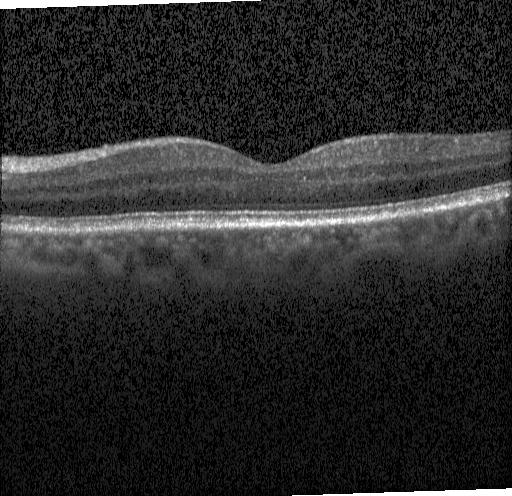

OCT B-scan · SD-OCT.
Impression: no evidence of CNV, DME, or drusen.